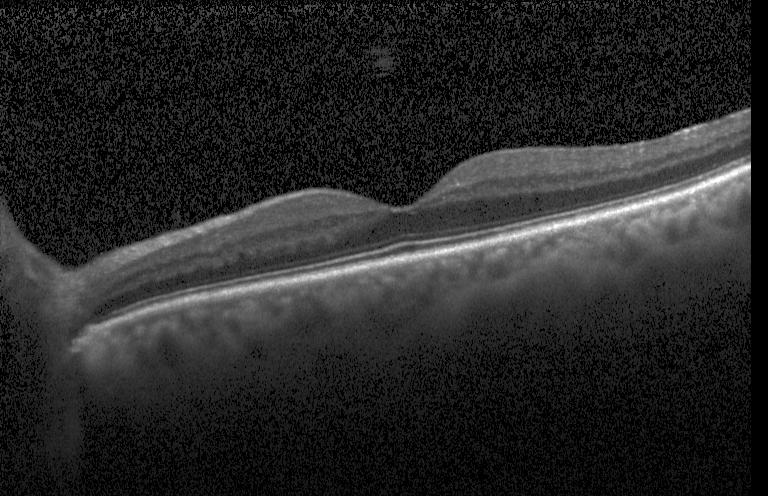

Horizontal scan through the fovea, Heidelberg Spectralis, OCT B-scan. Dx: no CNV, no DME, and no drusen.